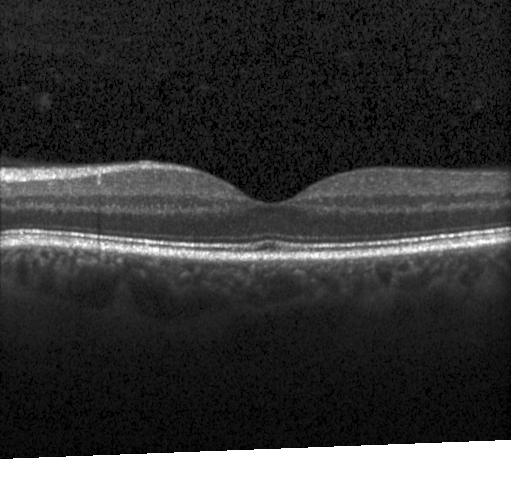 Macular scan; SD-OCT; retinal OCT B-scan; acquired on a Heidelberg Spectralis. Impression: neither choroidal neovascularization, diabetic macular edema, nor drusen.